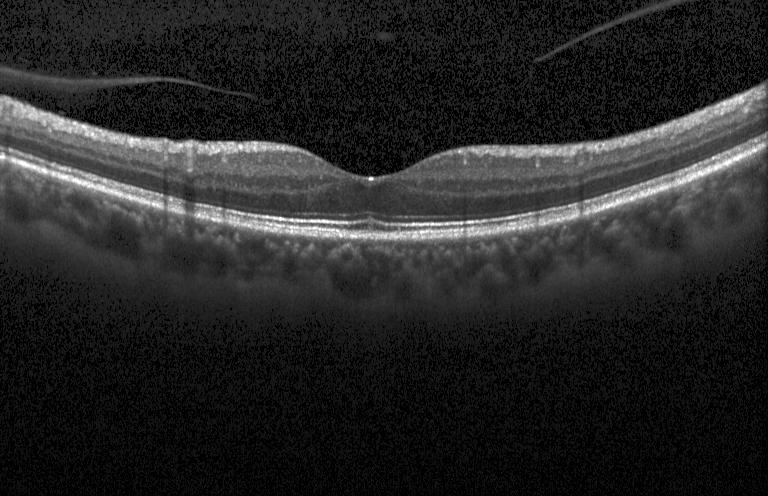 Macular OCT: no evidence of choroidal neovascularization, diabetic macular edema, or drusen.